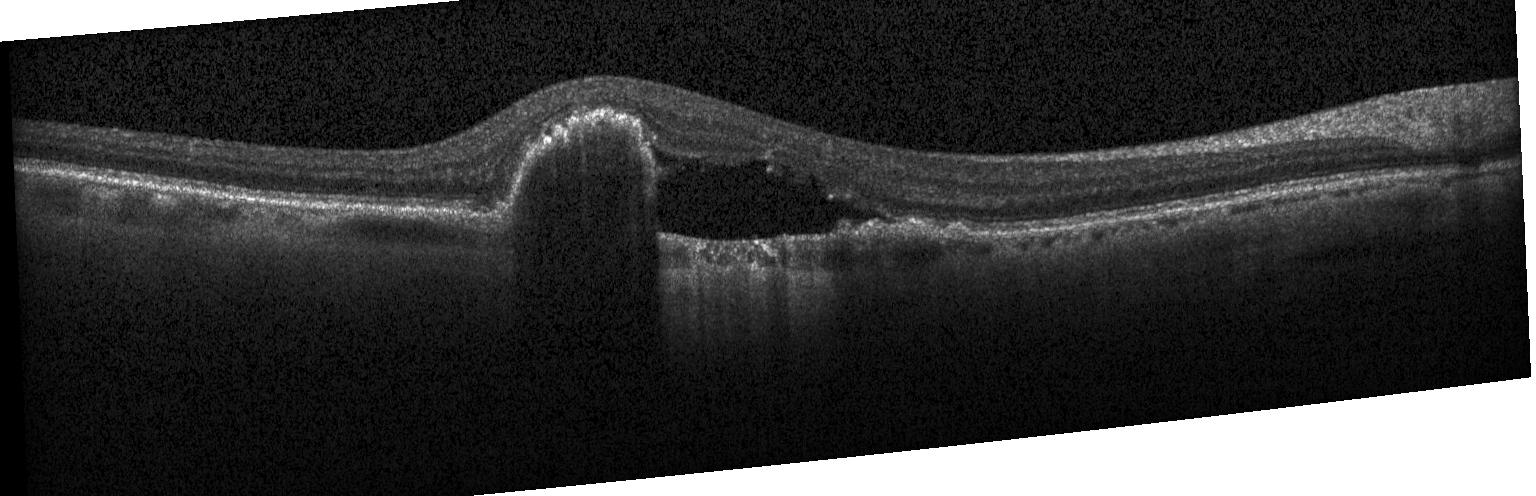 Macular scan · retinal OCT cross-section · spectral-domain OCT. Diagnosis: a choroidal neovascular membrane.